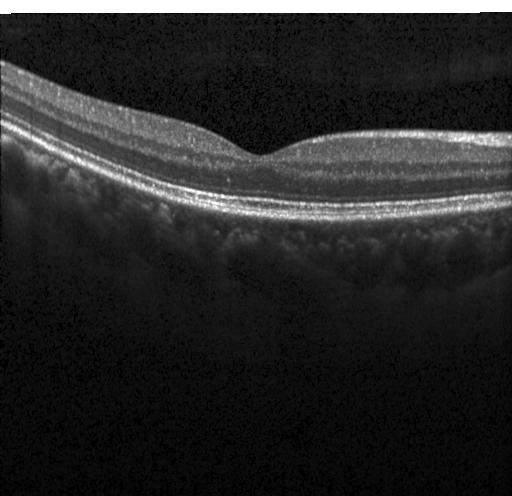
Retinal OCT cross-section. Heidelberg Spectralis OCT system
Macular OCT: no choroidal neovascularization, no diabetic macular edema, and no drusen.